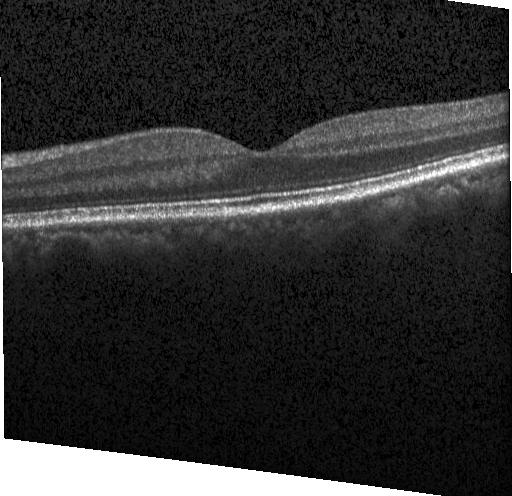
Retinal OCT cross-section
Macular OCT: no evidence of CNV, DME, or drusen.